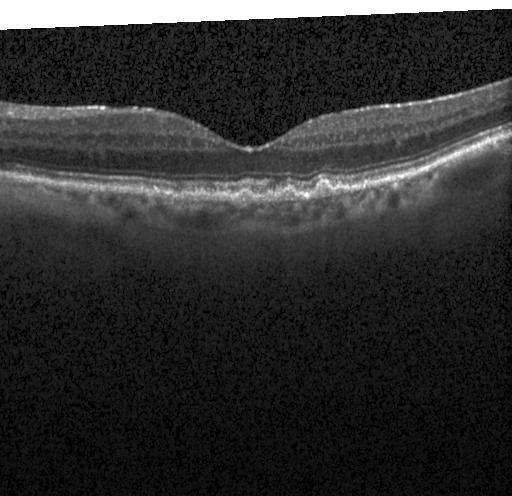

Impression: sub-RPE drusenoid deposits.